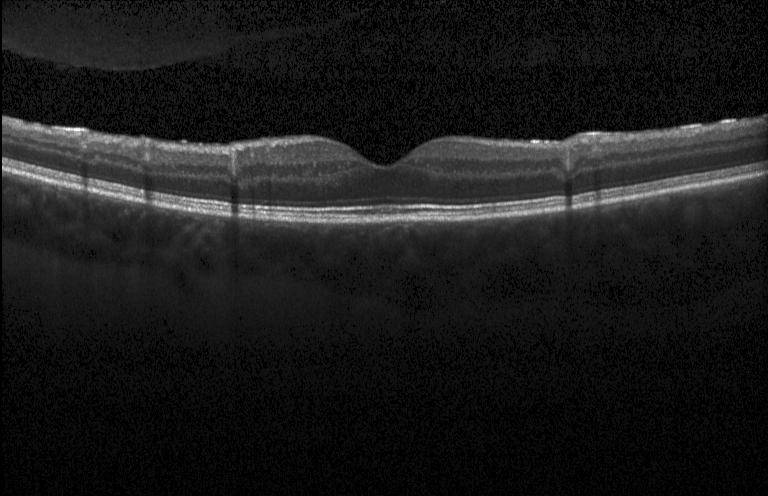

Diagnosis: neither CNV, DME, nor drusen.